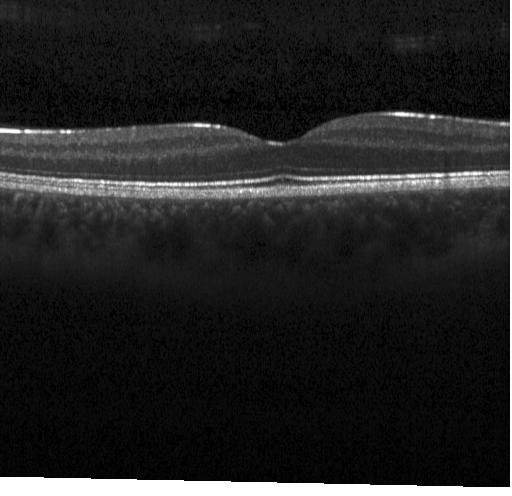

No CNV, DME, or drusen.